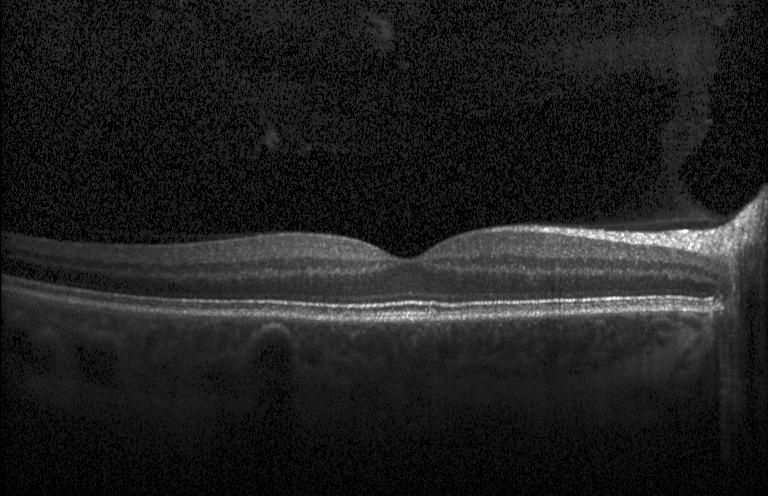

Macular OCT: no evidence of choroidal neovascularization, diabetic macular edema, or drusen.